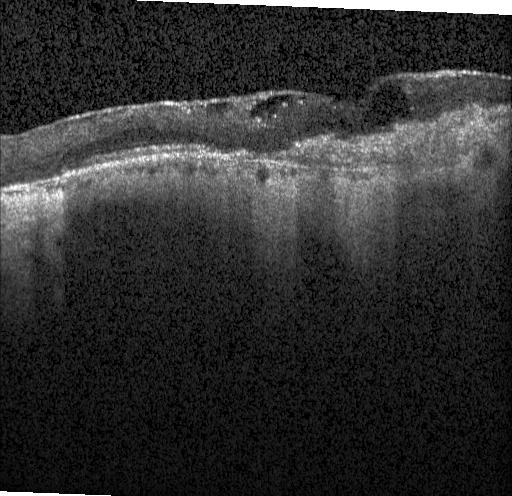
OCT B-scan showing a choroidal neovascular membrane.